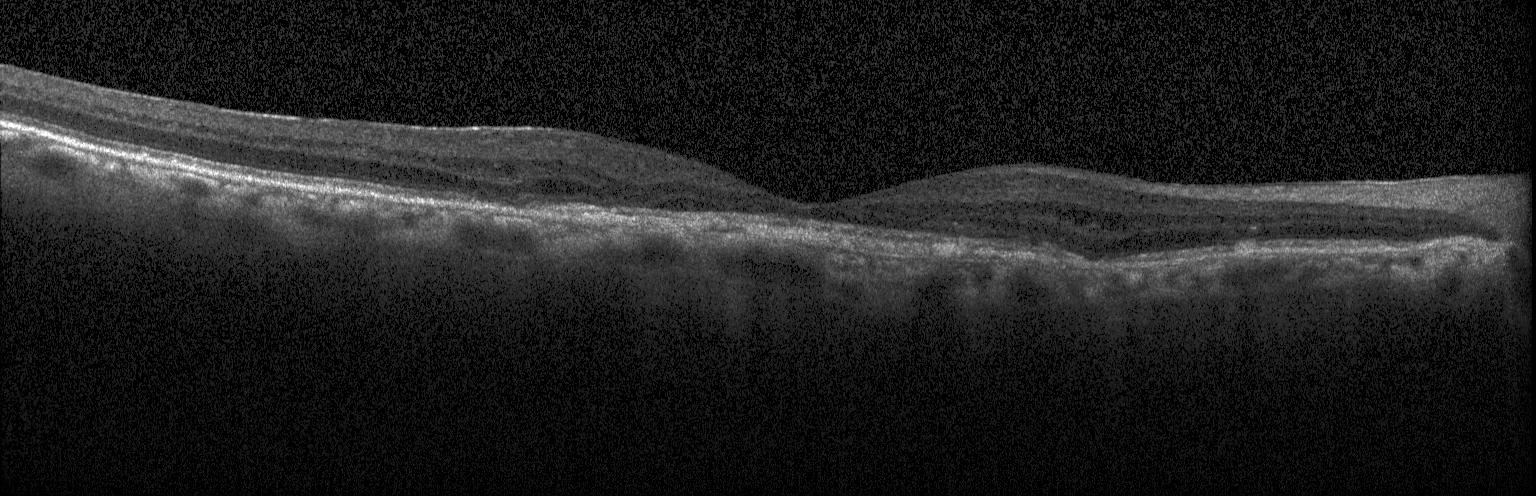

Fovea-centered; acquired on a Heidelberg Spectralis; SD-OCT; retinal OCT cross-section — The scan shows a choroidal neovascular membrane.